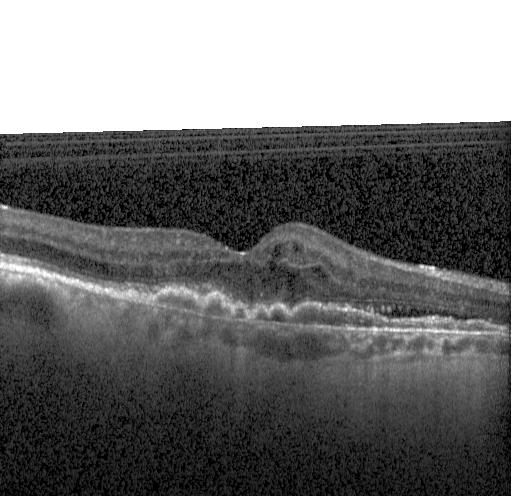 Heidelberg Spectralis, through the macula, OCT line scan
Impression: a choroidal neovascular membrane.